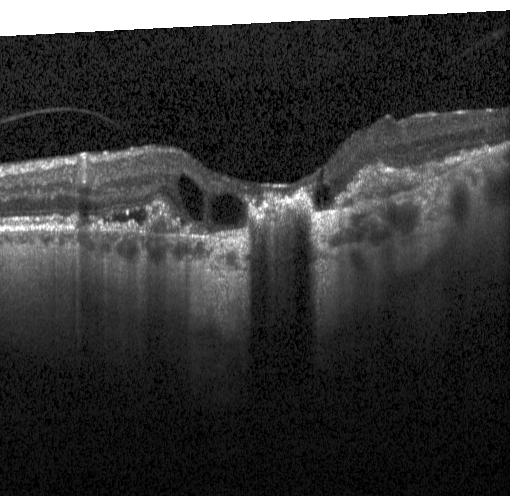

The scan shows CNV.